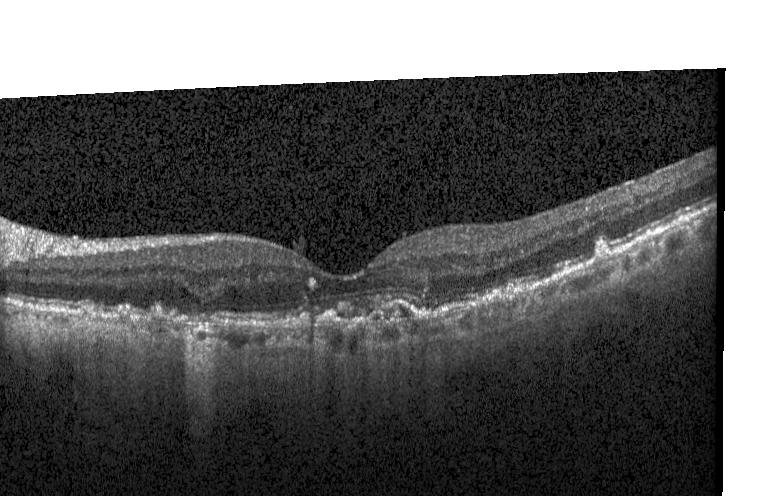
OCT B-scan. This B-scan demonstrates a choroidal neovascular membrane.